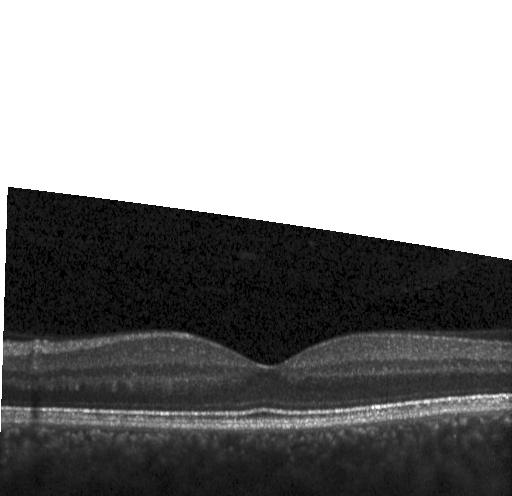

Optical coherence tomography B-scan. Assessment: no evidence of choroidal neovascularization, diabetic macular edema, or drusen.